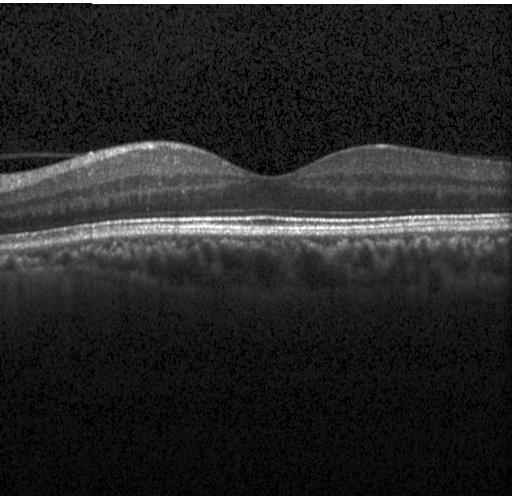
OCT line scan, centered on the fovea
Macular OCT: no choroidal neovascularization, no diabetic macular edema, and no drusen.